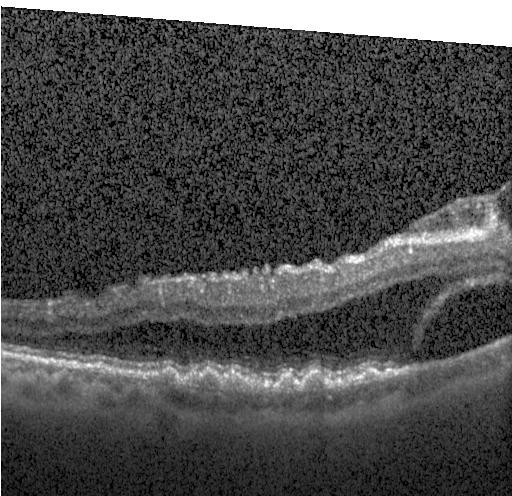
Heidelberg Spectralis, OCT line scan — Impression: choroidal neovascularization (CNV).